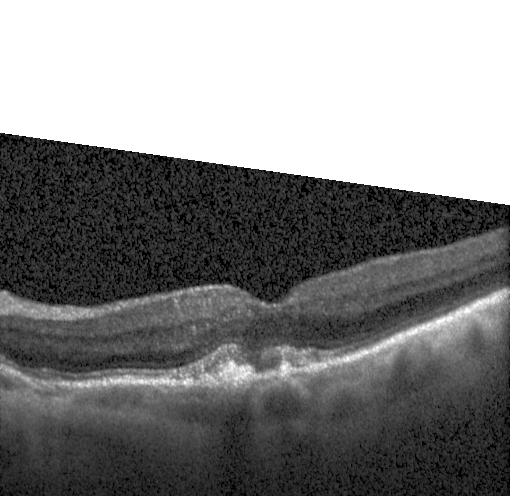 Retinal OCT cross-section, spectral-domain optical coherence tomography.
A choroidal neovascular membrane.